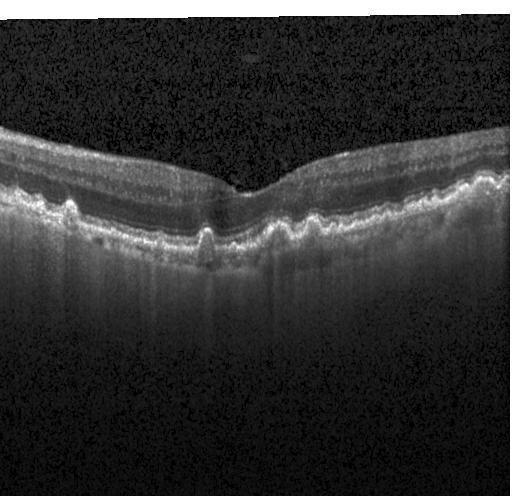
Impression: multiple drusen.